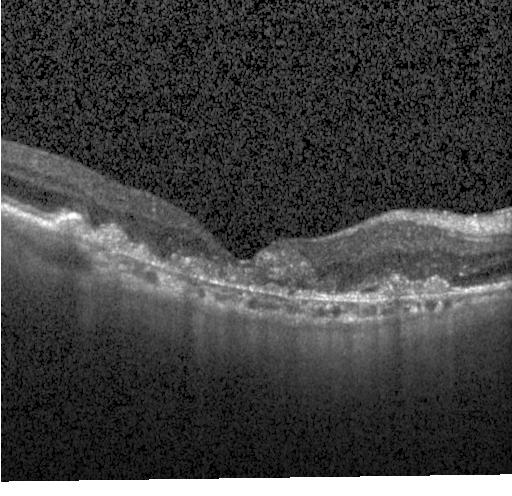 Centered on the fovea, SD-OCT, optical coherence tomography scan. Macular OCT: a choroidal neovascular membrane.